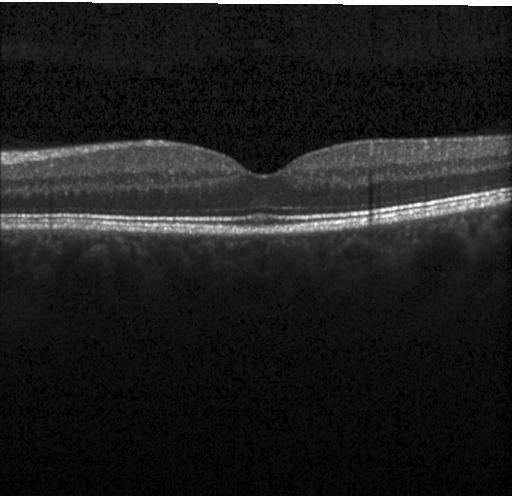
Retinal OCT B-scan, fovea-centered — Impression: neither CNV, DME, nor drusen.